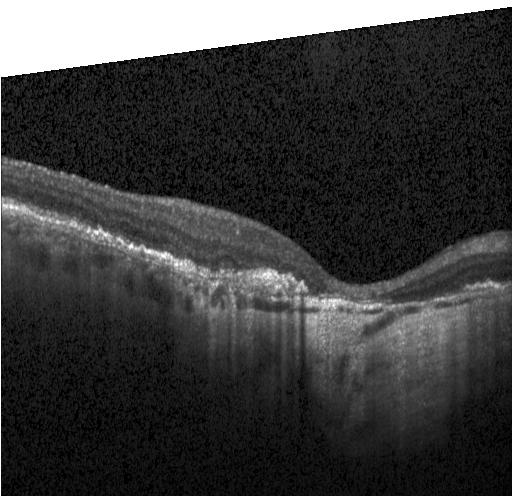
Retinal OCT B-scan — Finding: CNV.